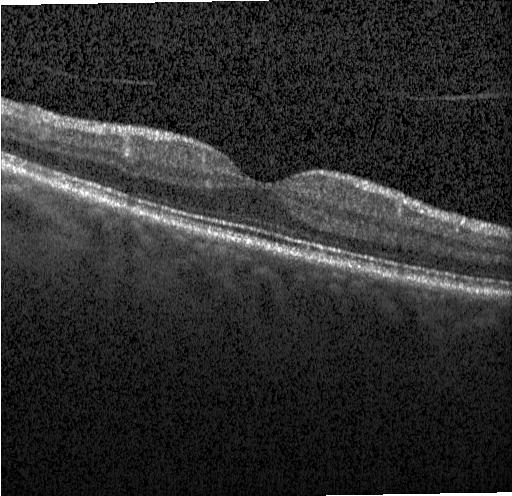 Impression: no evidence of choroidal neovascularization, diabetic macular edema, or drusen.